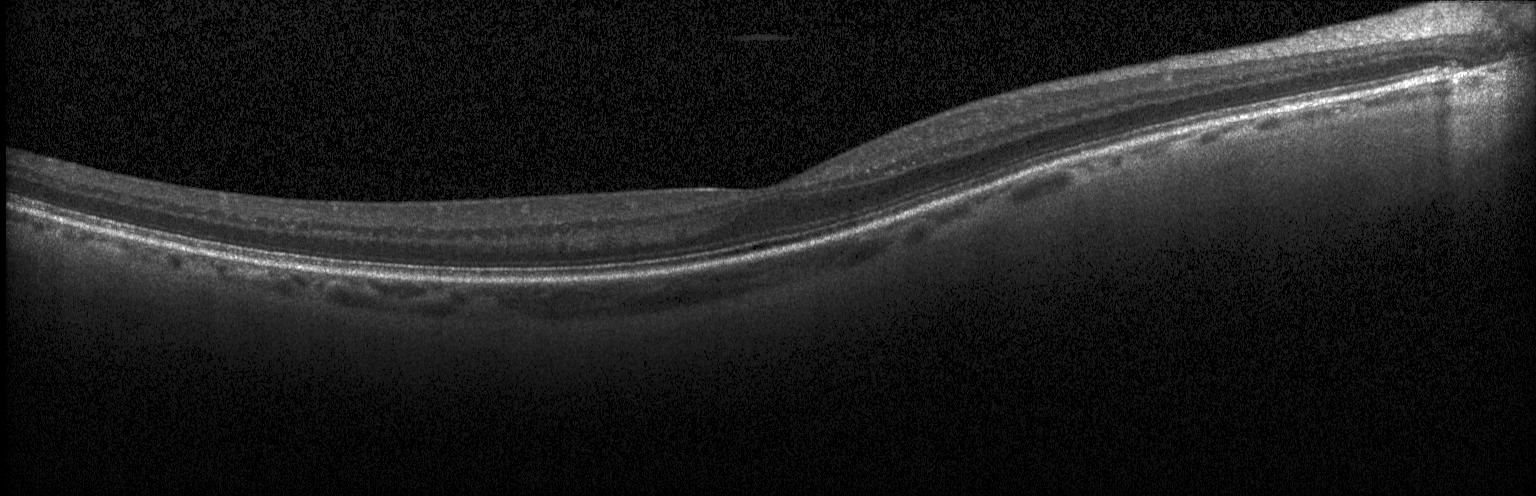 Spectral-domain OCT, OCT B-scan. OCT finding: no evidence of choroidal neovascularization, diabetic macular edema, or drusen.